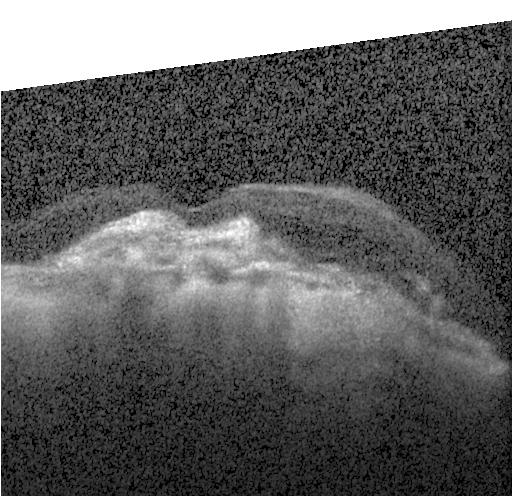
Spectral-domain OCT; retinal OCT cross-section; fovea-centered; instrument: Heidelberg Spectralis
A choroidal neovascular membrane.